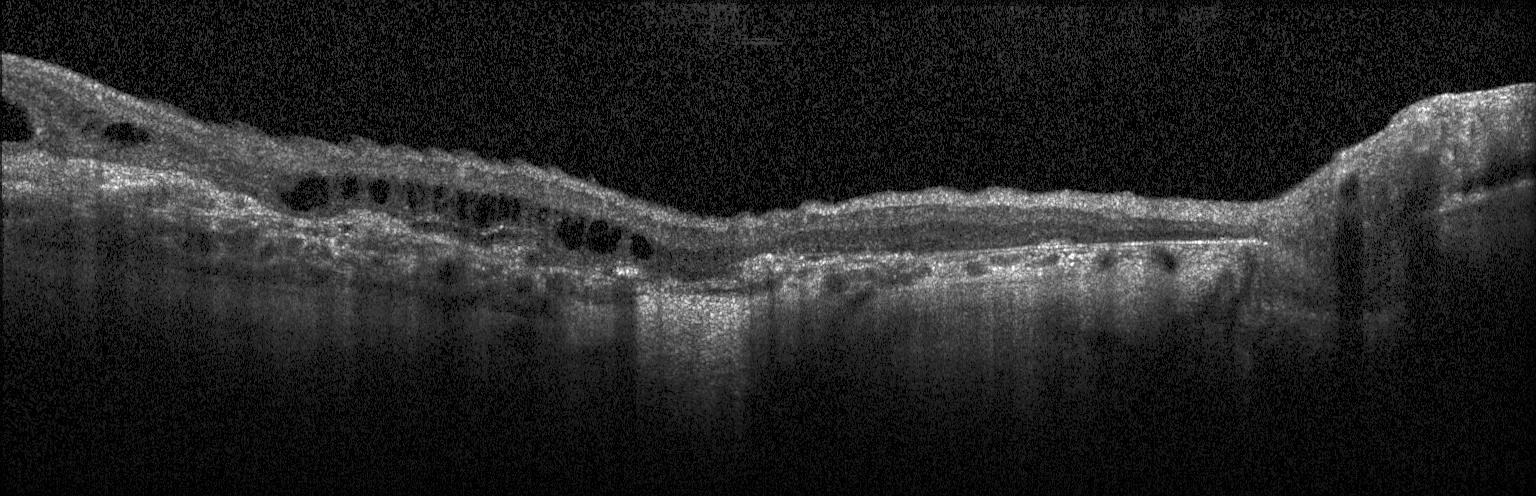
Fovea-centered · OCT B-scan — This B-scan demonstrates a choroidal neovascular membrane.